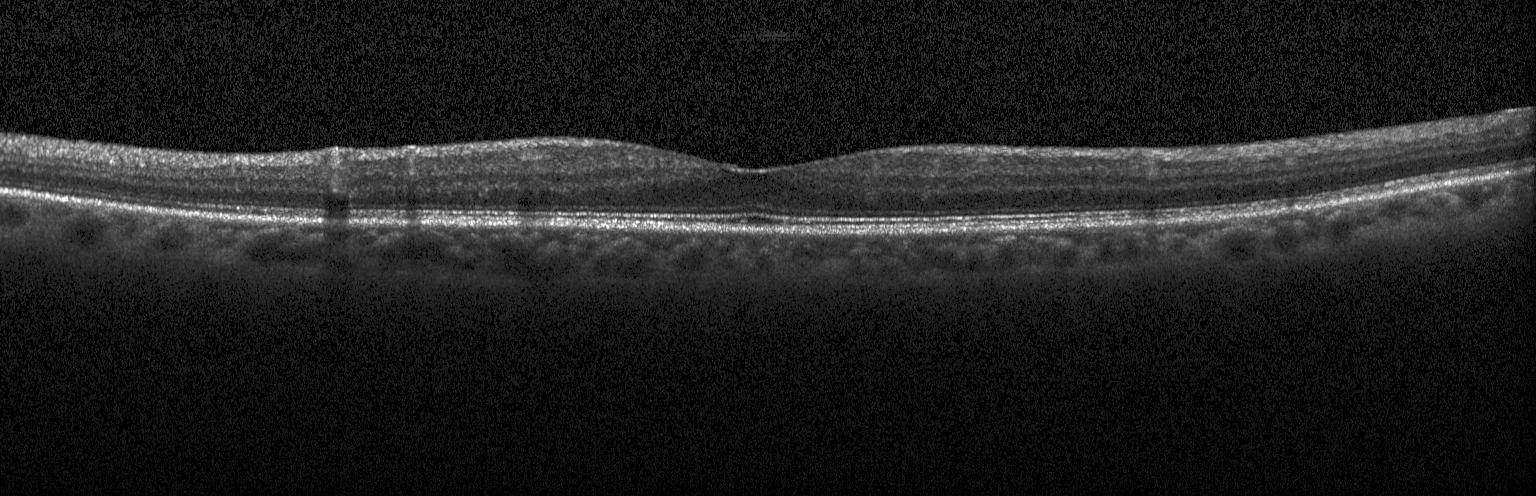
Impression: no choroidal neovascularization, no diabetic macular edema, and no drusen.